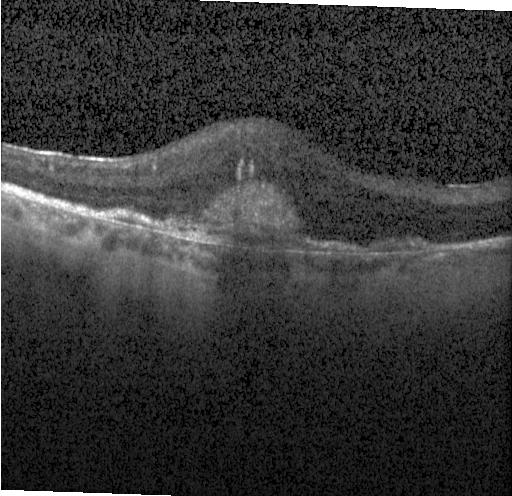
Choroidal neovascularization.